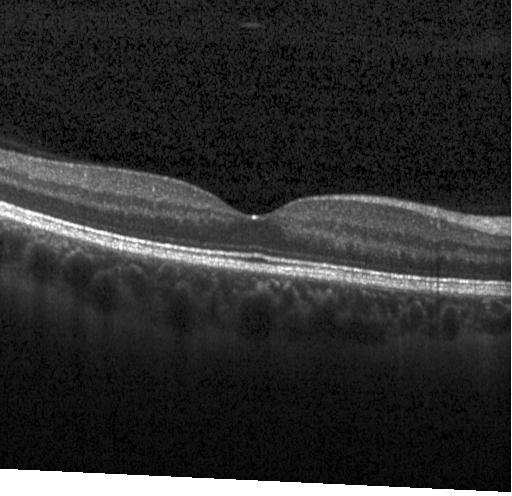
OCT B-scan. Macular OCT: no evidence of CNV, DME, or drusen.